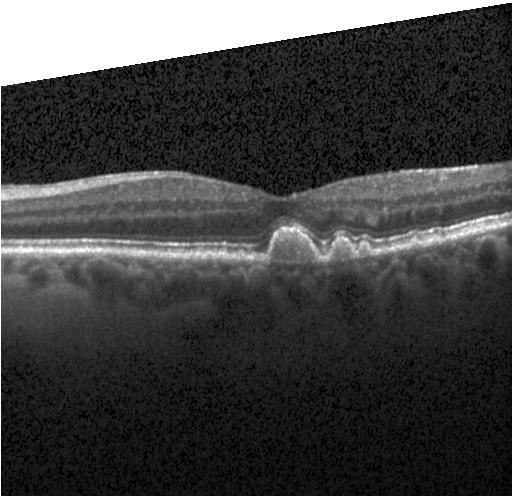

Retinal OCT B-scan · macular scan.
Assessment: multiple drusen.